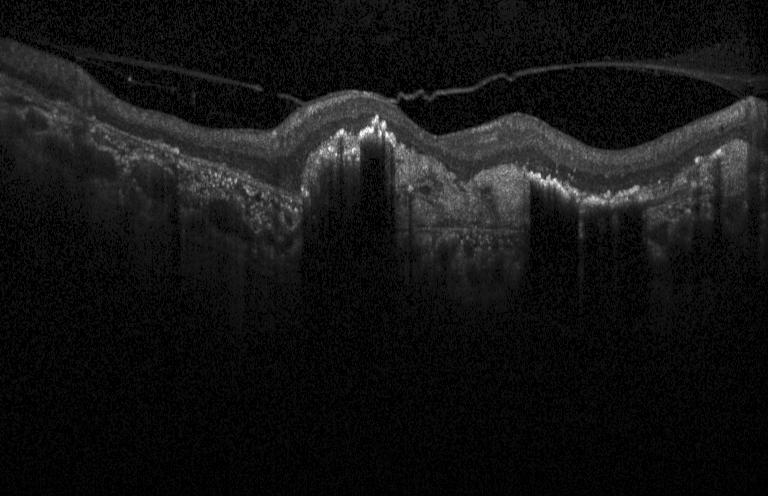 Finding: a choroidal neovascular membrane.